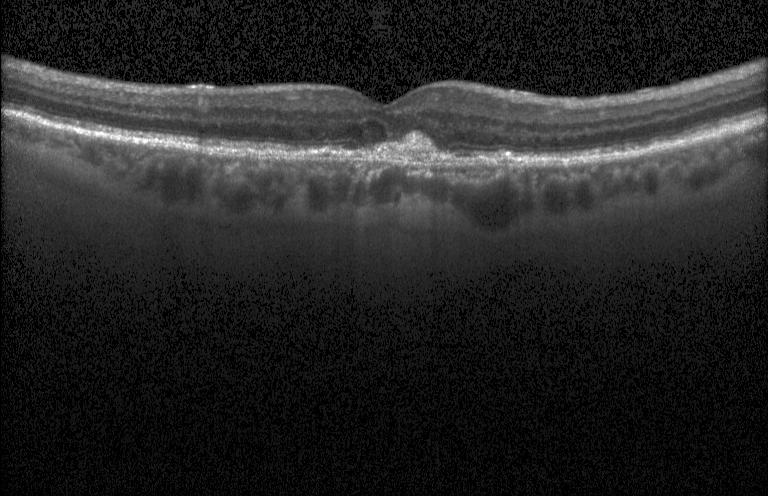 Macular scan. Retinal OCT cross-section. SD-OCT. Heidelberg Spectralis OCT system — Diagnosis: choroidal neovascularization (CNV).